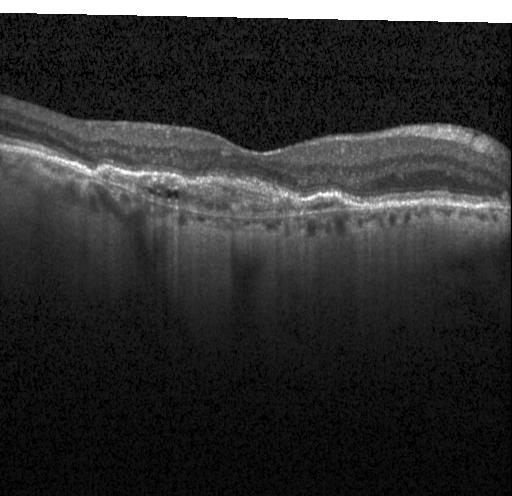
SD-OCT · optical coherence tomography scan · horizontal scan through the fovea.
Macular OCT: choroidal neovascularization (CNV).